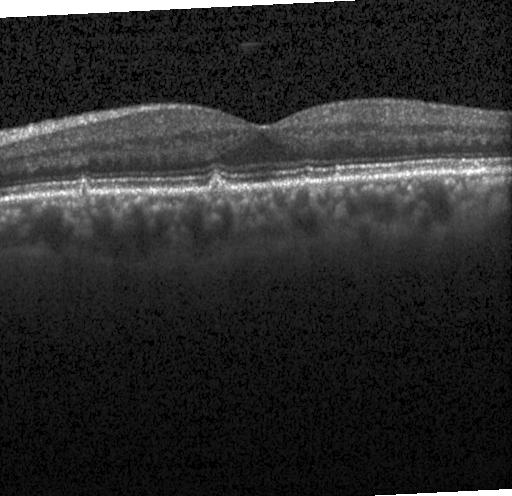 Optical coherence tomography B-scan; through the macula; Heidelberg Spectralis
Dx: sub-RPE drusenoid deposits.